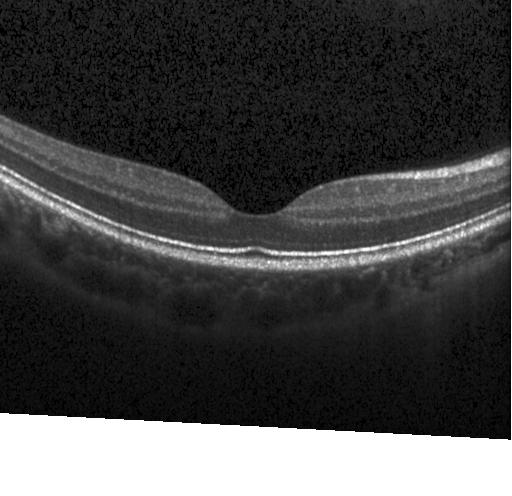

Macular scan. Spectral-domain OCT. OCT B-scan.
Neither CNV, DME, nor drusen.